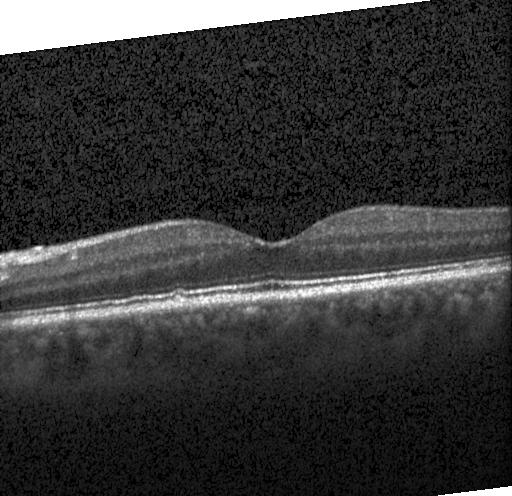 OCT line scan · Heidelberg Spectralis OCT system · macular scan
Finding: drusen.